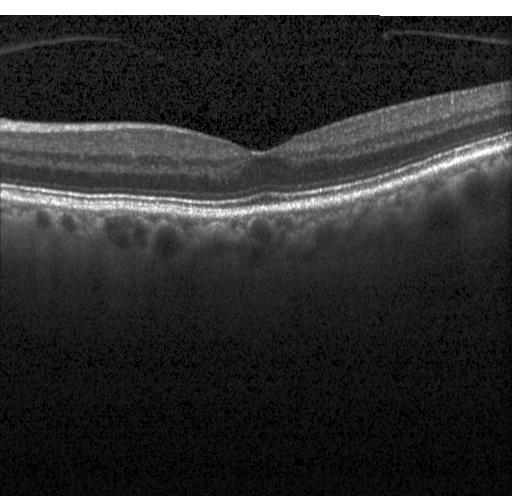
Heidelberg Spectralis, optical coherence tomography B-scan, through the macula.
Dx: no choroidal neovascularization, no diabetic macular edema, and no drusen.